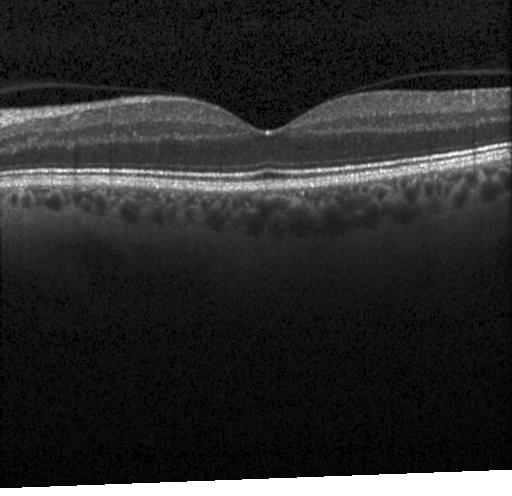
Impression: no choroidal neovascularization, no diabetic macular edema, and no drusen.